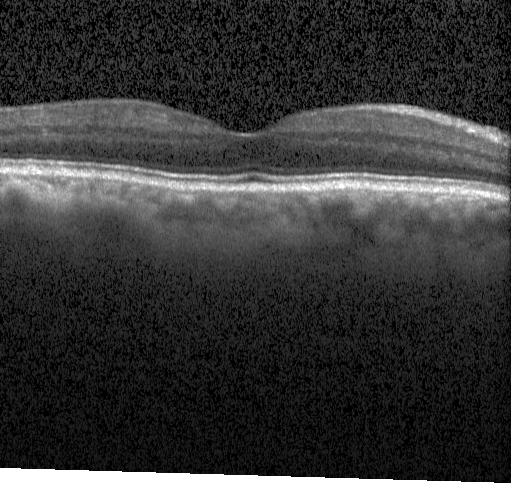
Fovea-centered · OCT line scan
Macular OCT: no choroidal neovascularization, no diabetic macular edema, and no drusen.